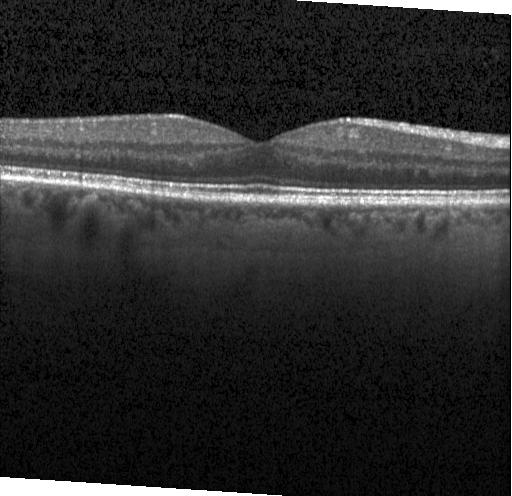

Retinal OCT B-scan; Heidelberg Spectralis.
Dx: no choroidal neovascularization, no diabetic macular edema, and no drusen.